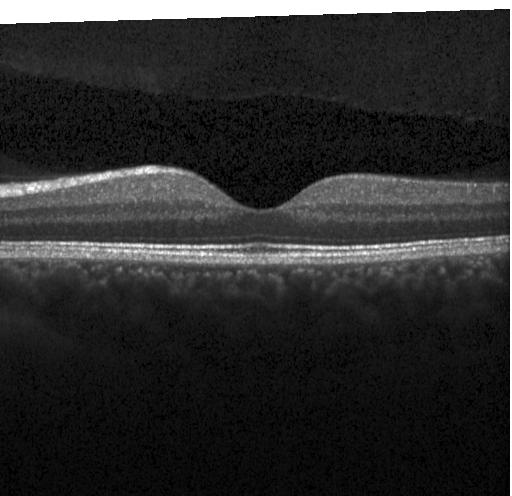

Retinal OCT cross-section, spectral-domain optical coherence tomography, acquired on a Heidelberg Spectralis
Diagnosis: no choroidal neovascularization, no diabetic macular edema, and no drusen.